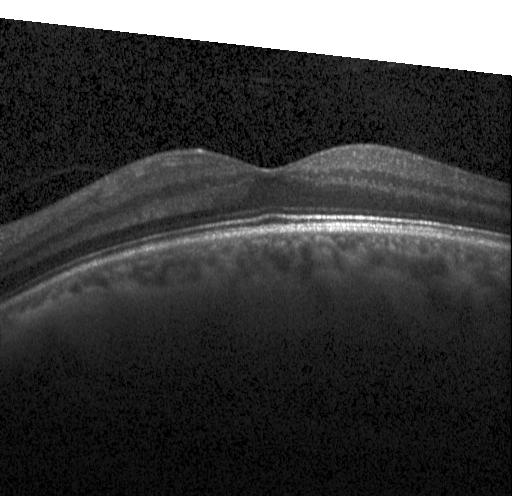 Spectral-domain OCT B-scan: no choroidal neovascularization, no diabetic macular edema, and no drusen.